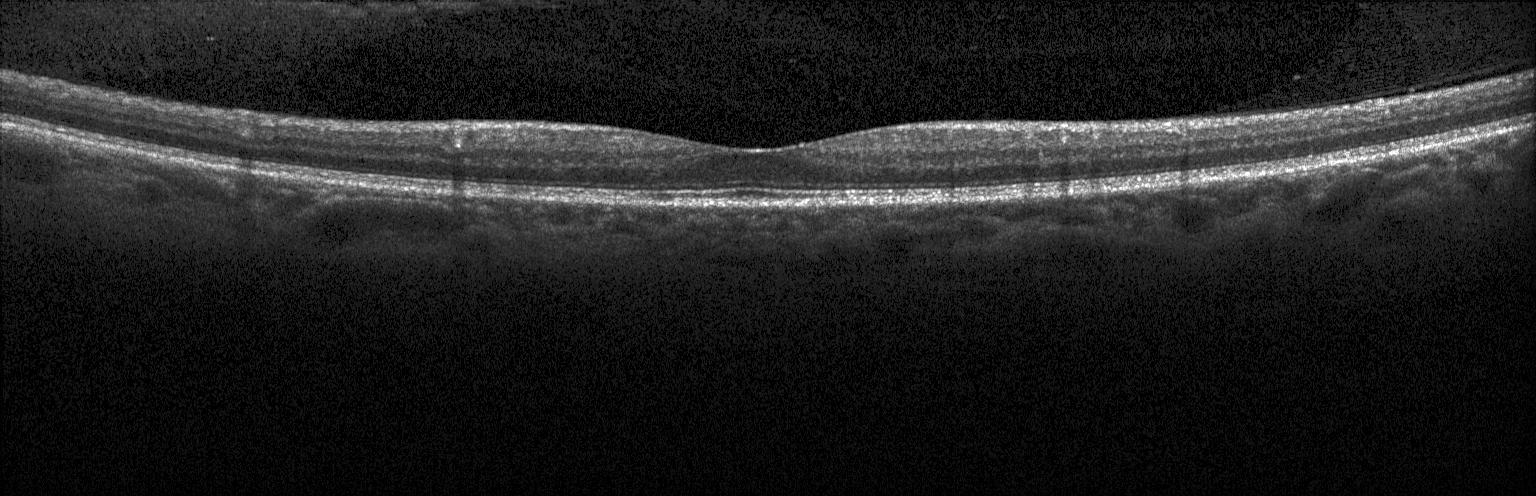
Optical coherence tomography scan
Impression: no evidence of CNV, DME, or drusen.